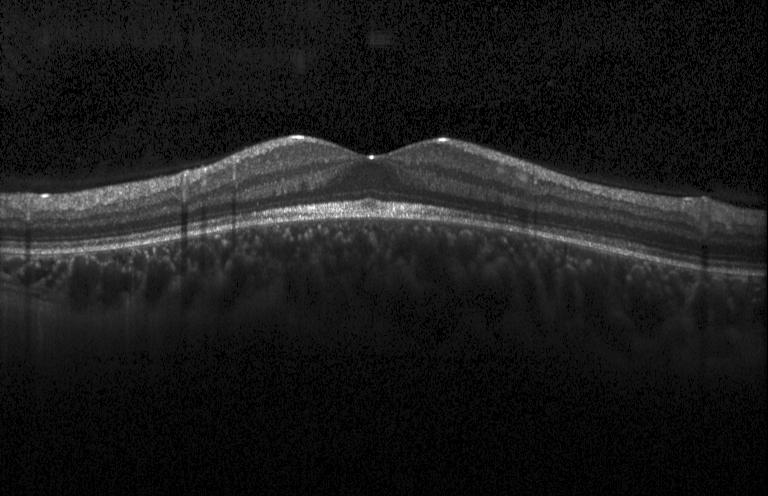

Centered on the fovea. SD-OCT. OCT B-scan — No choroidal neovascularization, no diabetic macular edema, and no drusen.